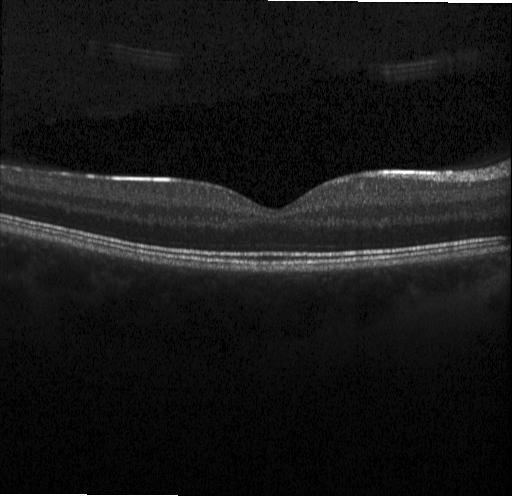
OCT B-scan; instrument: Heidelberg Spectralis; through the macula — Finding: no CNV, no DME, and no drusen.